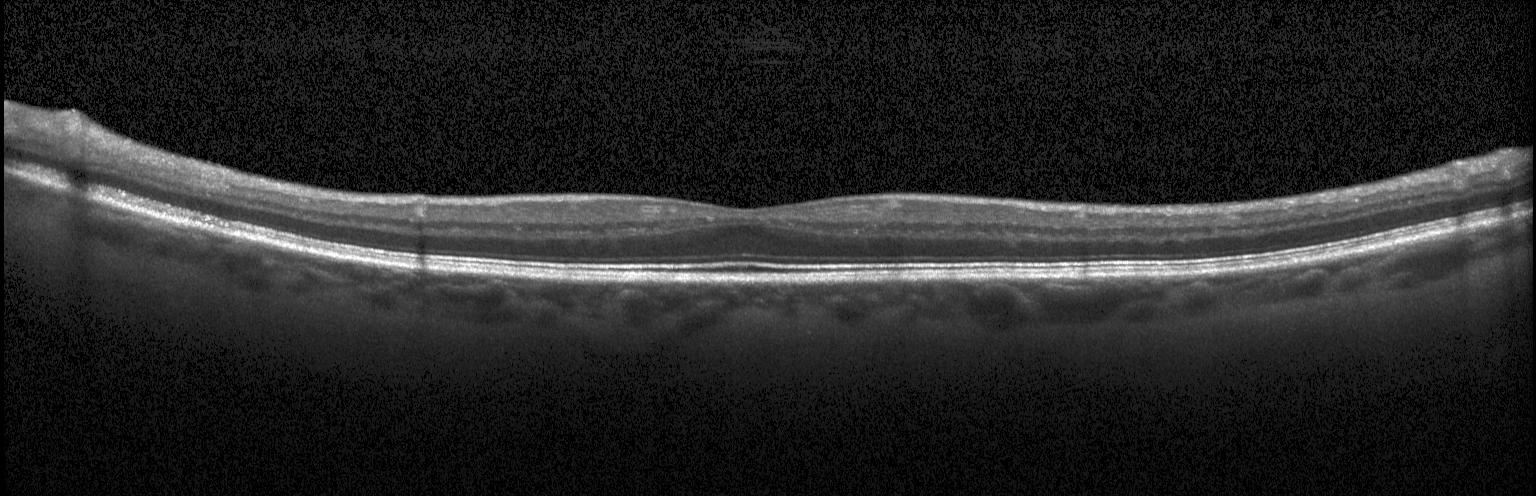
OCT finding: no choroidal neovascularization, diabetic macular edema, or drusen.